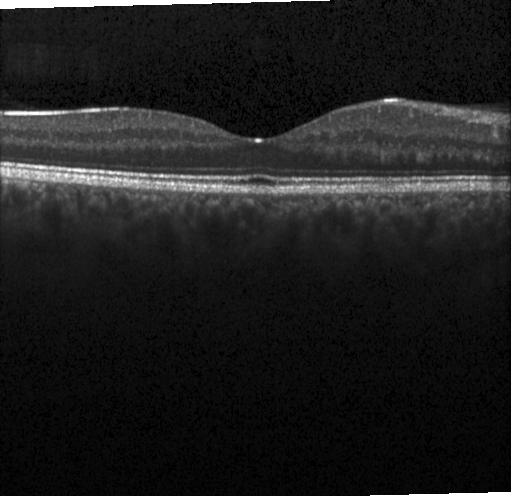

SD-OCT, Heidelberg Spectralis OCT system, OCT B-scan.
Dx: no choroidal neovascularization, diabetic macular edema, or drusen.